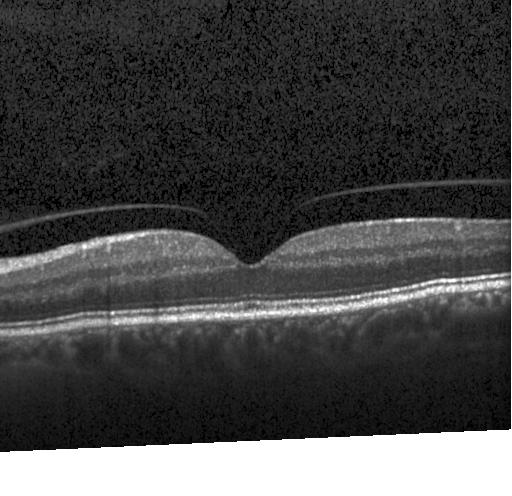 Finding: no choroidal neovascularization, no diabetic macular edema, and no drusen.